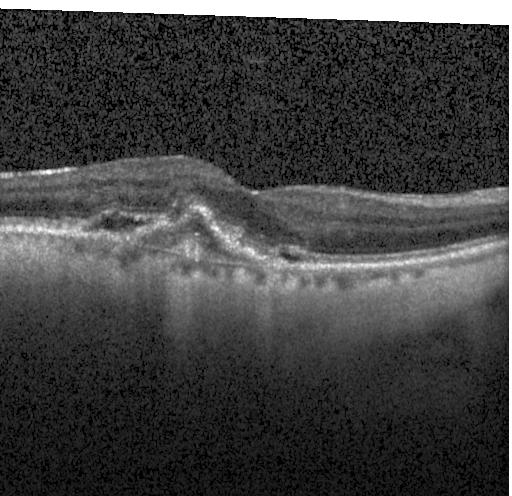

OCT line scan. Acquired on a Heidelberg Spectralis. SD-OCT. Macular OCT: CNV.